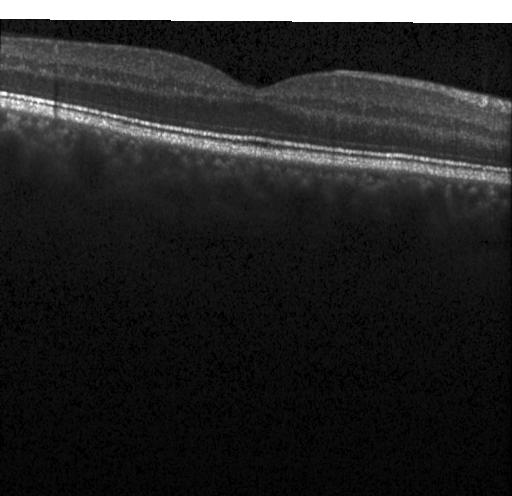

Neither choroidal neovascularization, diabetic macular edema, nor drusen.